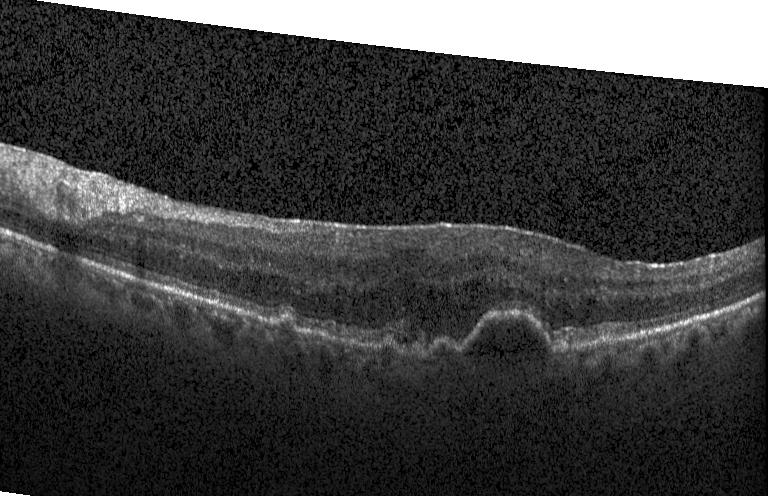
The scan shows a choroidal neovascular membrane.